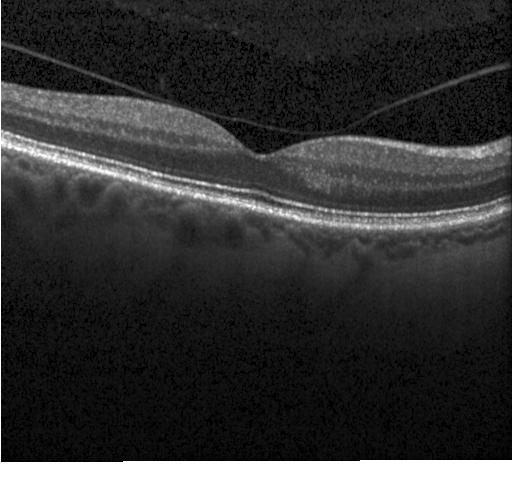
Through the macula, optical coherence tomography scan, SD-OCT
Diagnosis: no choroidal neovascularization, no diabetic macular edema, and no drusen.